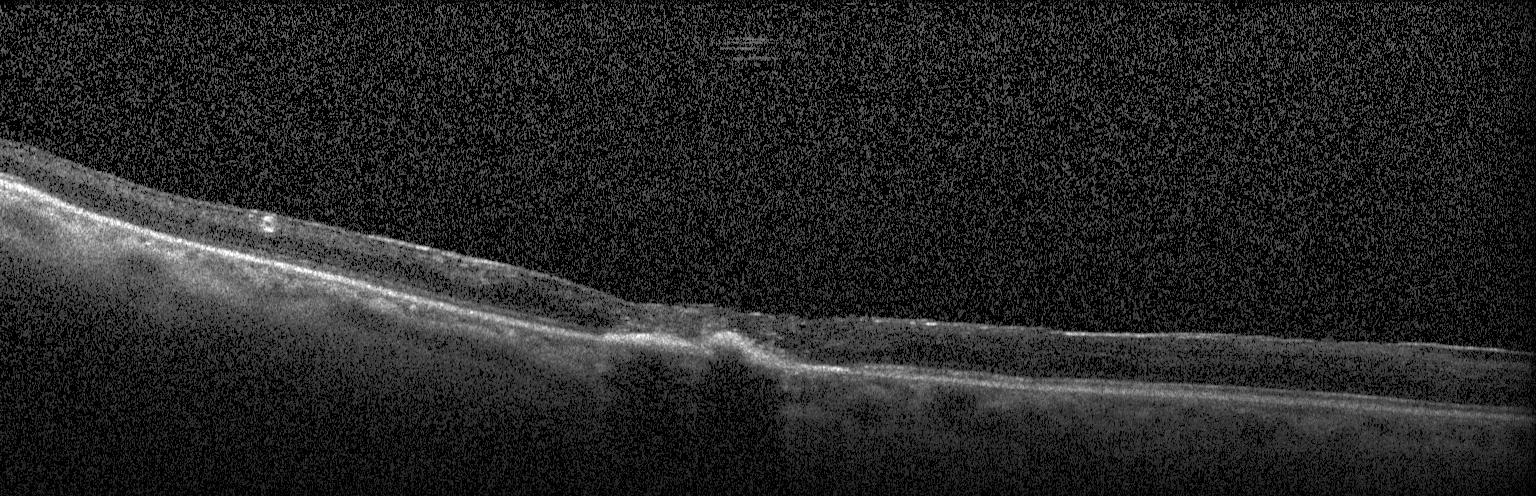
OCT B-scan showing a choroidal neovascular membrane.